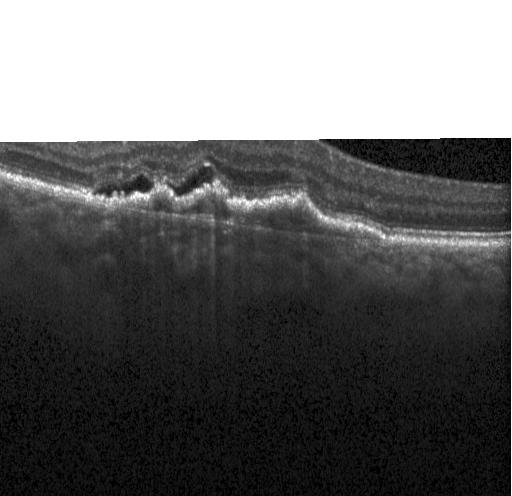
Impression: a choroidal neovascular membrane.